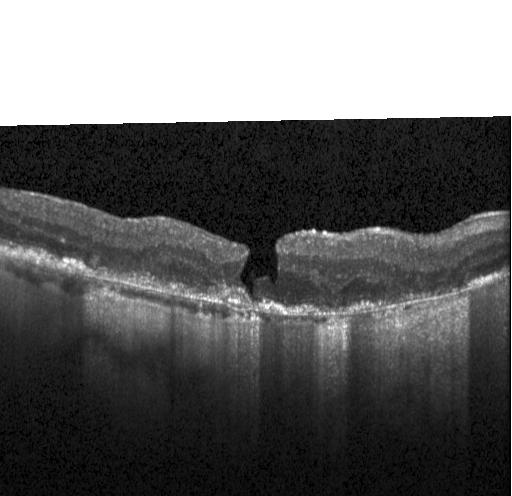

Macular OCT demonstrating a choroidal neovascular membrane.